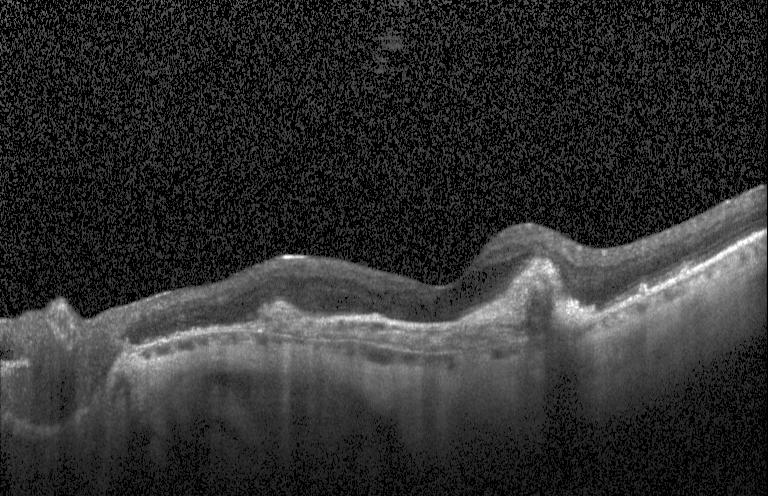 Retinal OCT B-scan; Heidelberg Spectralis OCT system.
Diagnosis: a choroidal neovascular membrane.